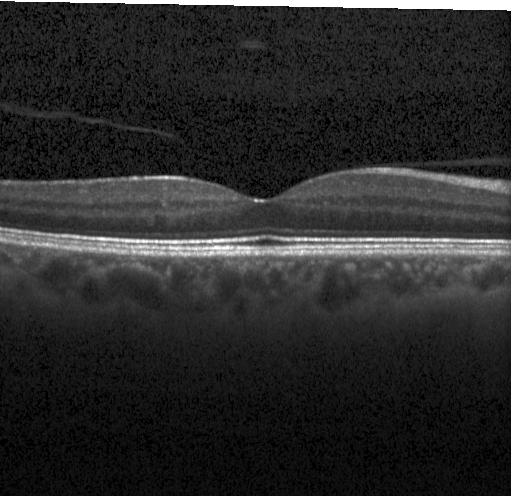
Instrument: Heidelberg Spectralis, macular scan, OCT B-scan.
Dx: neither CNV, DME, nor drusen.